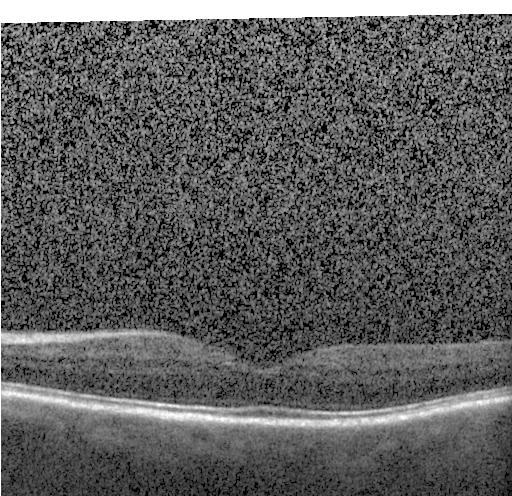

Optical coherence tomography scan — Diagnosis: no choroidal neovascularization, no diabetic macular edema, and no drusen.